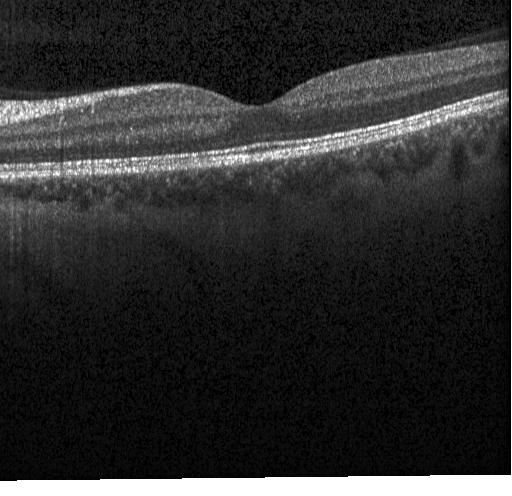

OCT B-scan, centered on the fovea — The scan shows no choroidal neovascularization, no diabetic macular edema, and no drusen.